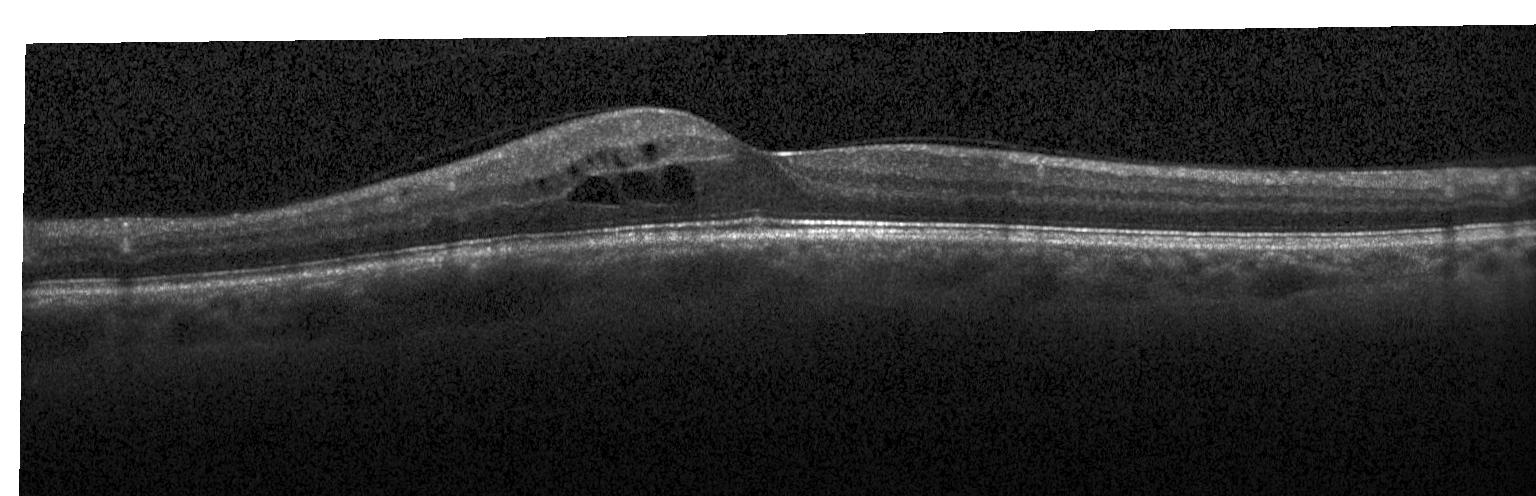
OCT B-scan · spectral-domain OCT.
Finding: diabetic macular edema (DME).